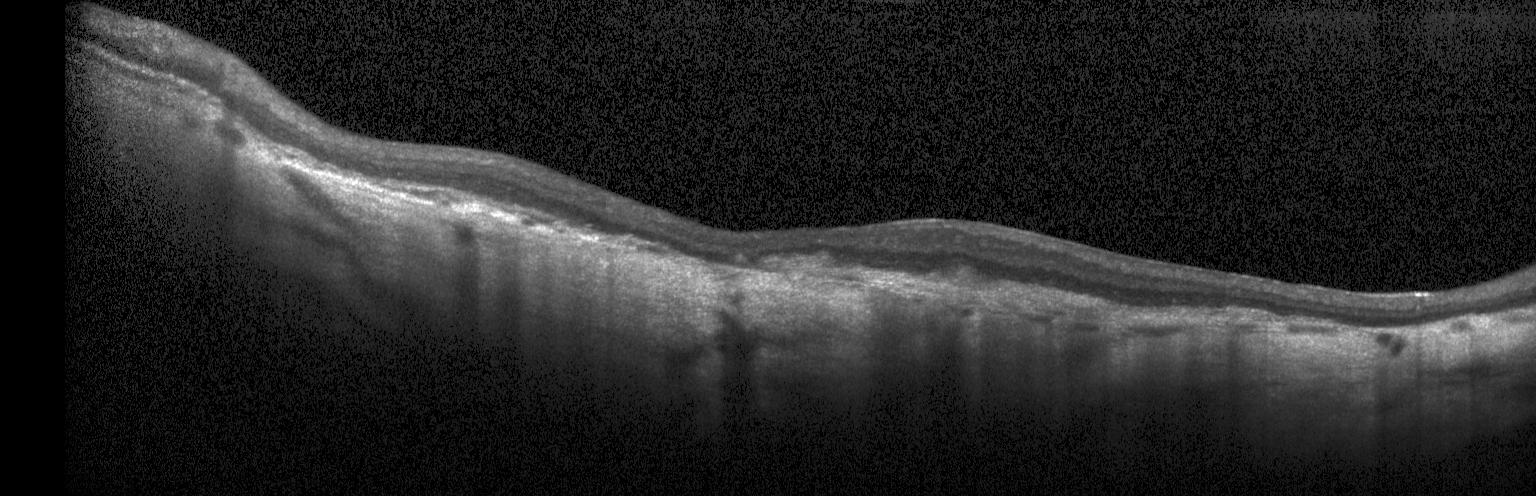
Optical coherence tomography B-scan
Dx: a choroidal neovascular membrane.